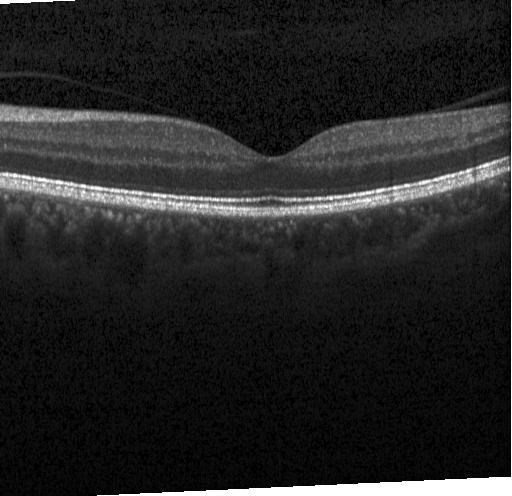 OCT B-scan showing no choroidal neovascularization, no diabetic macular edema, and no drusen.